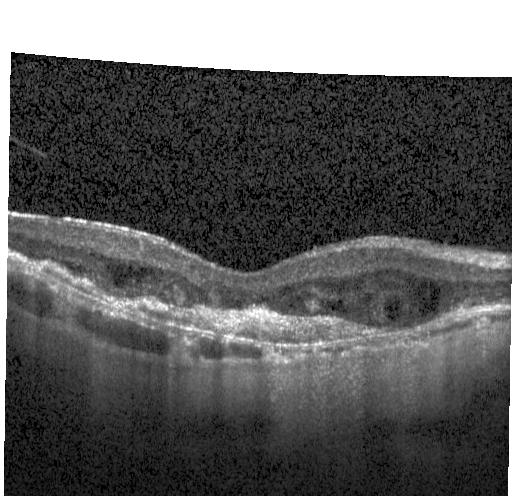
OCT B-scan — Diagnosis: CNV.